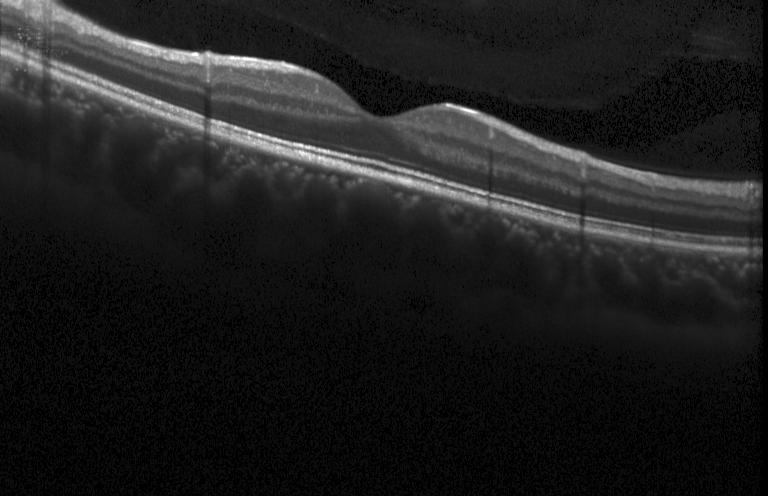
OCT line scan. Spectral-domain optical coherence tomography — Diagnosis: no choroidal neovascularization, diabetic macular edema, or drusen.